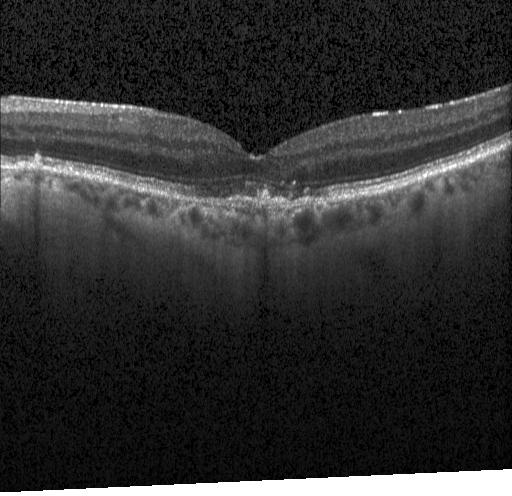 Acquired on a Heidelberg Spectralis, OCT line scan, fovea-centered. Dx: choroidal neovascularization (CNV).